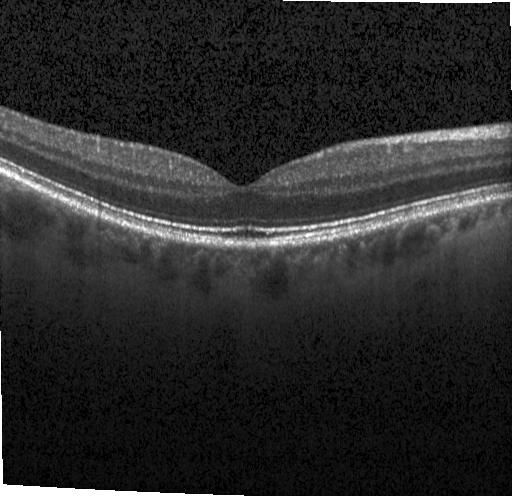

Horizontal scan through the fovea; OCT B-scan.
No CNV, DME, or drusen.